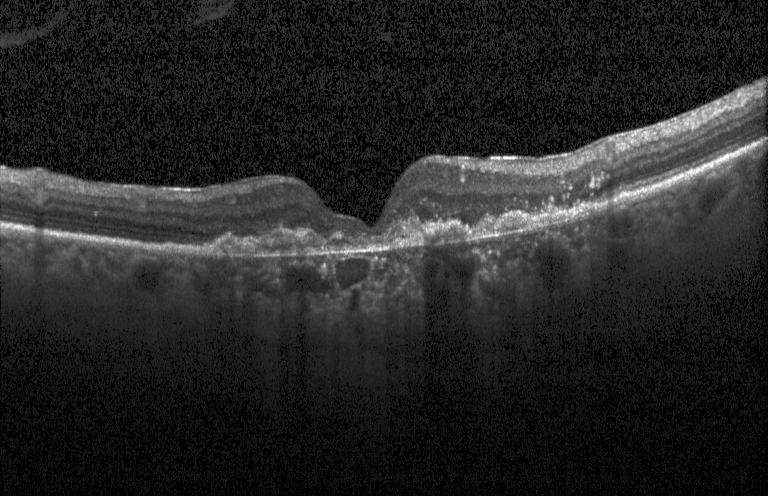 Dx: a choroidal neovascular membrane.